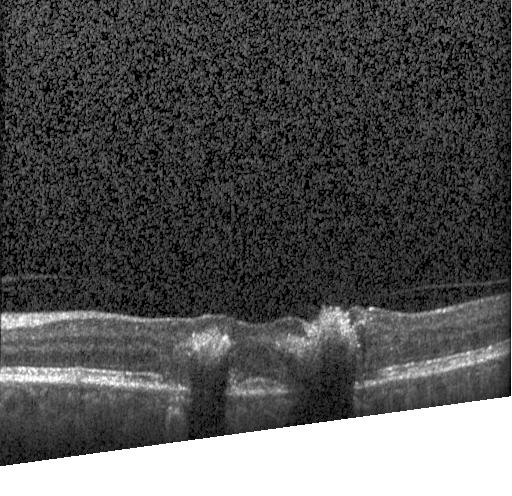
Diagnosis: a choroidal neovascular membrane.